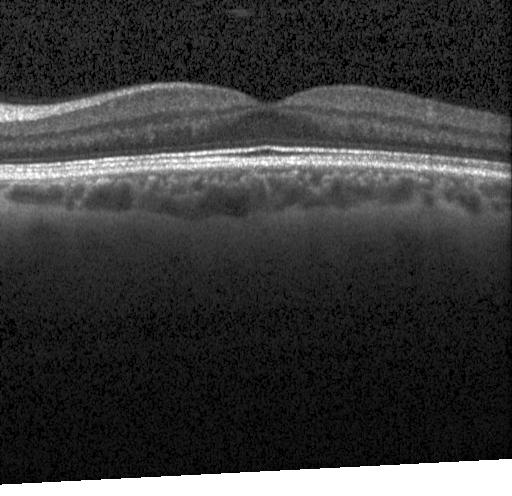 Retinal OCT cross-section, acquired on a Heidelberg Spectralis, spectral-domain optical coherence tomography, macular scan — This B-scan demonstrates neither CNV, DME, nor drusen.